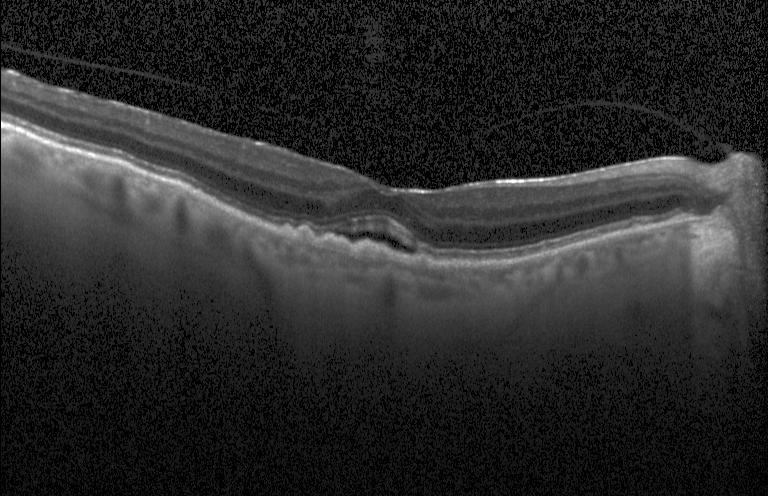
Optical coherence tomography scan; spectral-domain OCT
OCT finding: a choroidal neovascular membrane.